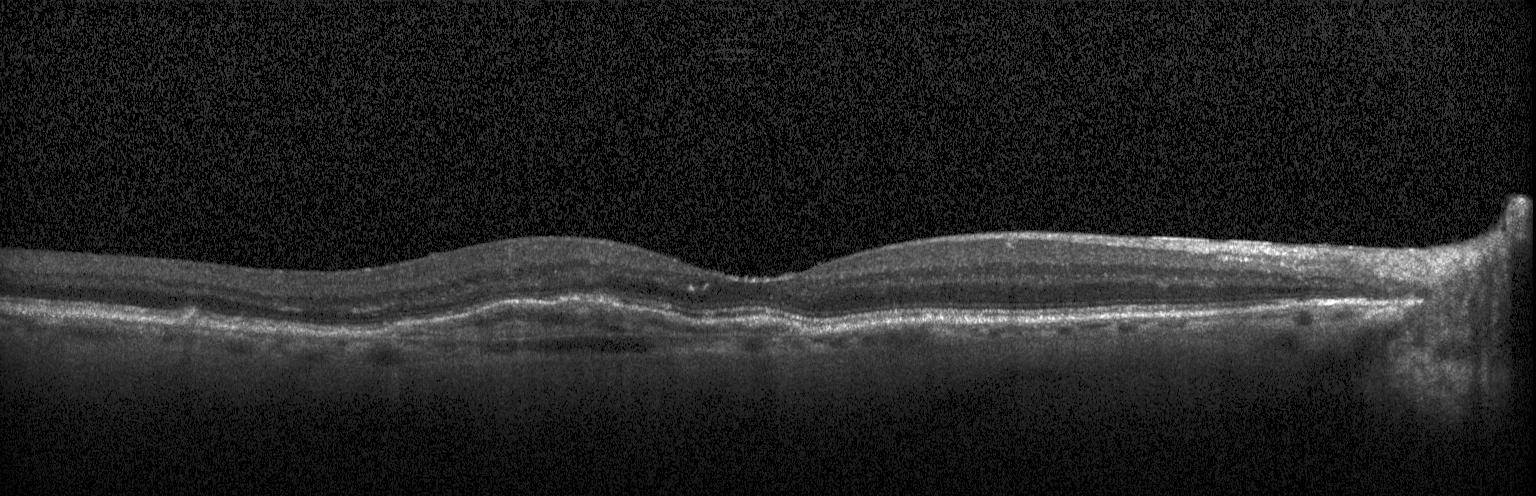
Macular OCT demonstrating a choroidal neovascular membrane.